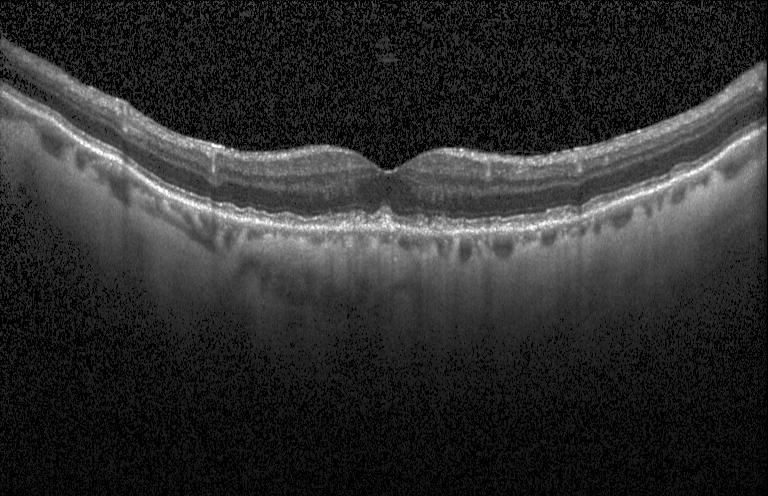
Centered on the fovea · optical coherence tomography B-scan · SD-OCT — Impression: sub-RPE drusenoid deposits.